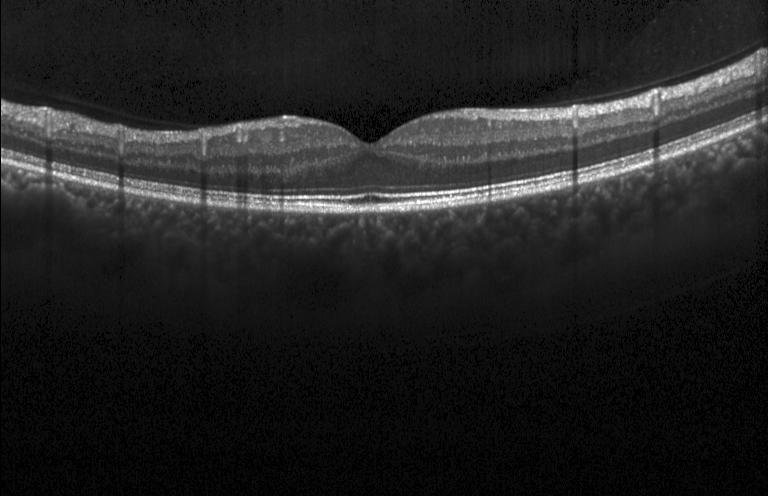 This B-scan demonstrates no choroidal neovascularization, diabetic macular edema, or drusen.